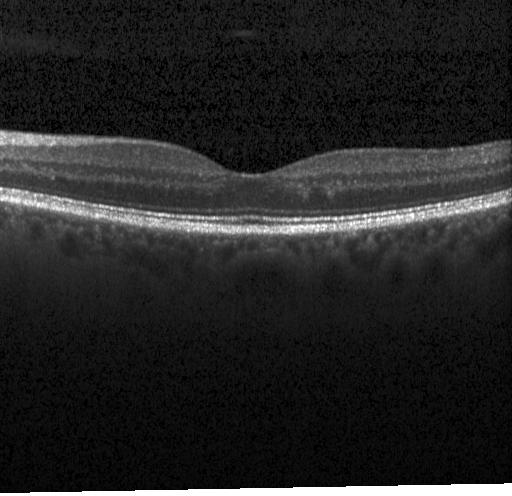

Finding: no CNV, DME, or drusen.